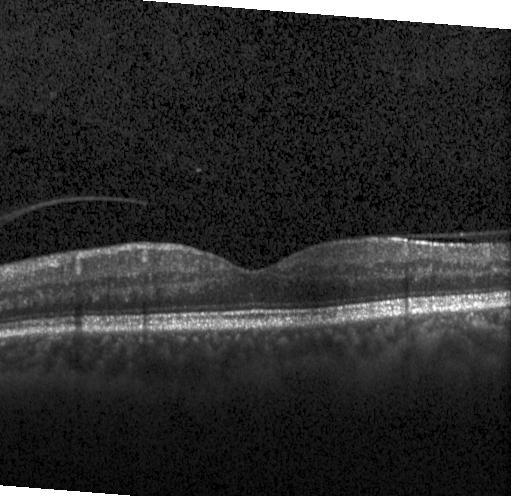
Macular OCT: no evidence of choroidal neovascularization, diabetic macular edema, or drusen.